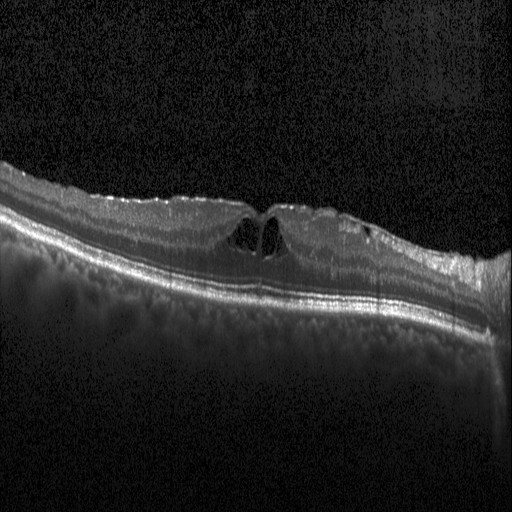

Assessment: diabetic macular edema (DME).